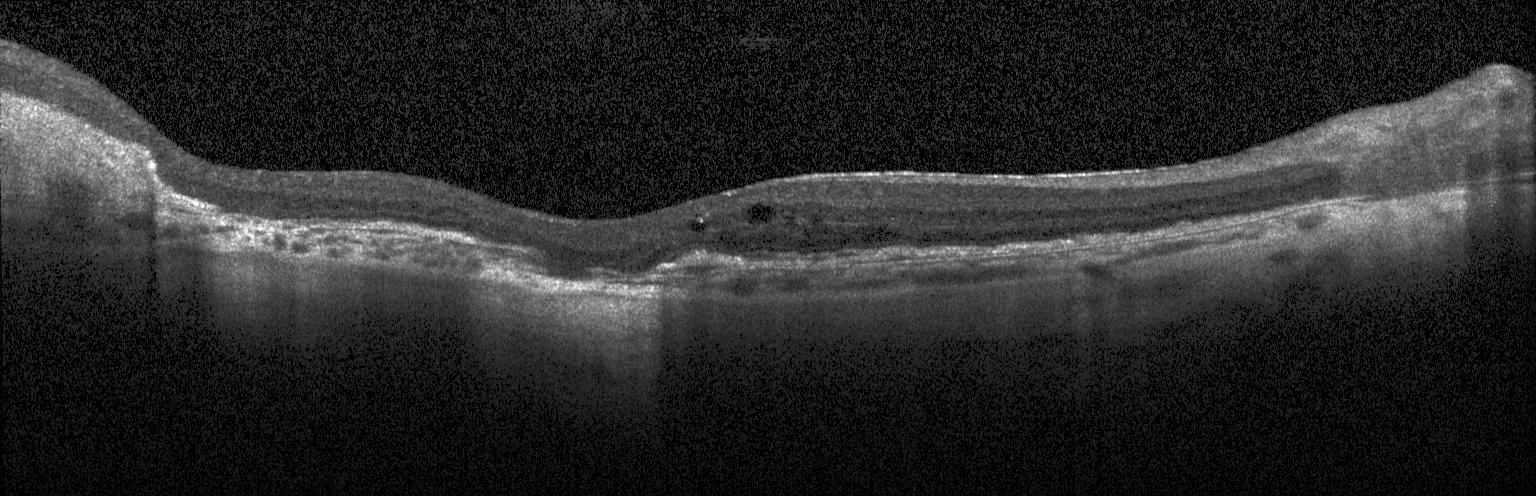

Retinal OCT cross-section. Dx: a choroidal neovascular membrane.